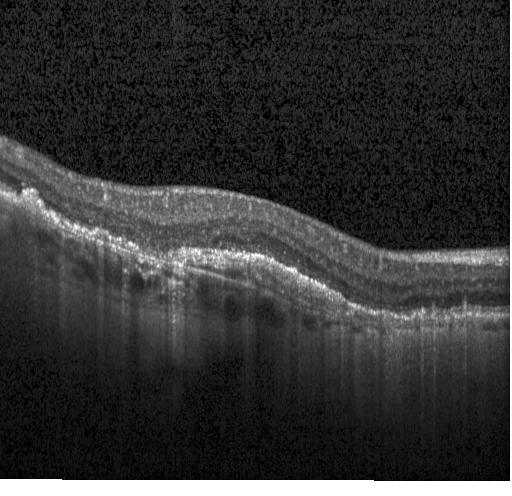

Horizontal scan through the fovea. Spectral-domain OCT. Optical coherence tomography B-scan.
Macular OCT: choroidal neovascularization (CNV).